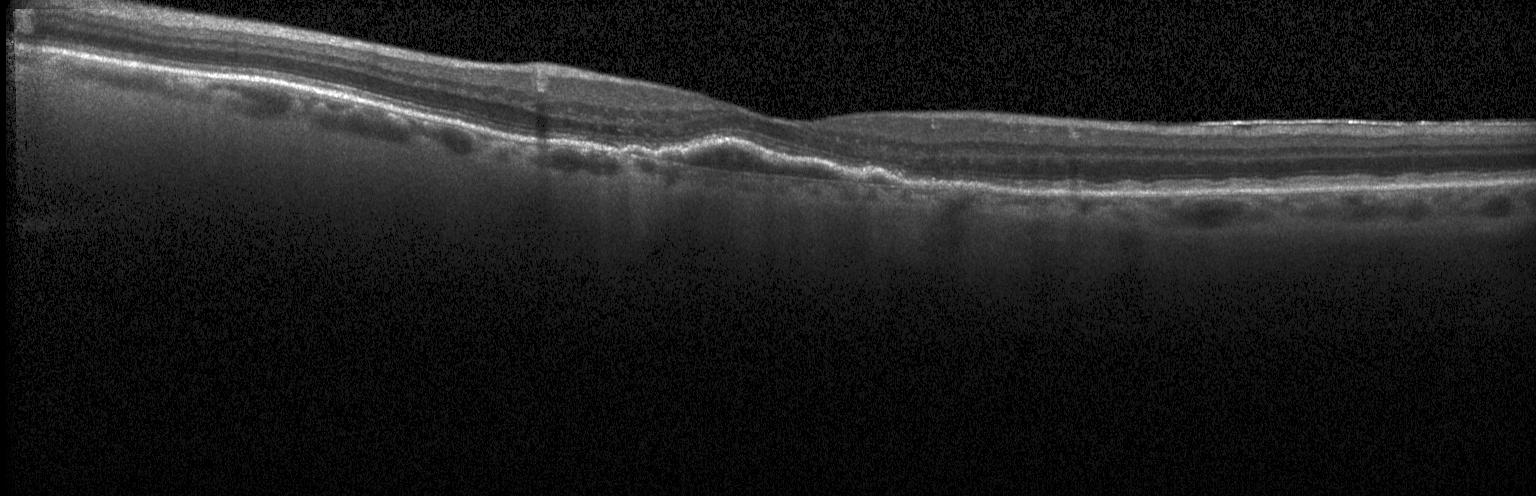
OCT finding: a choroidal neovascular membrane.